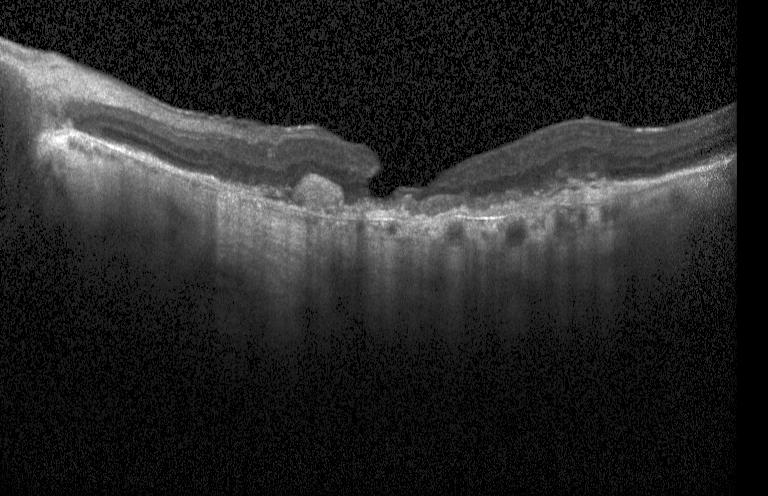
Through the macula. Spectral-domain optical coherence tomography. Optical coherence tomography B-scan. Heidelberg Spectralis. The scan shows choroidal neovascularization.